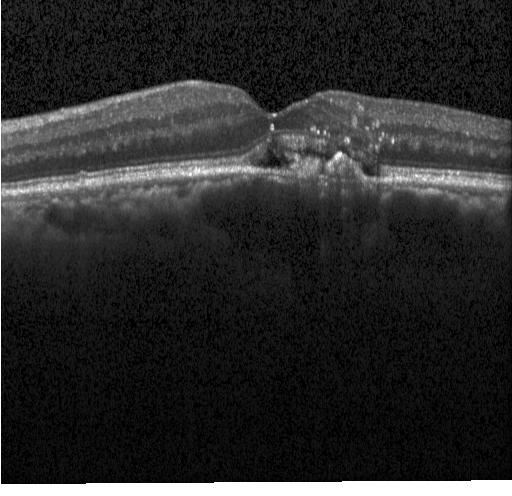 Dx: a choroidal neovascular membrane.